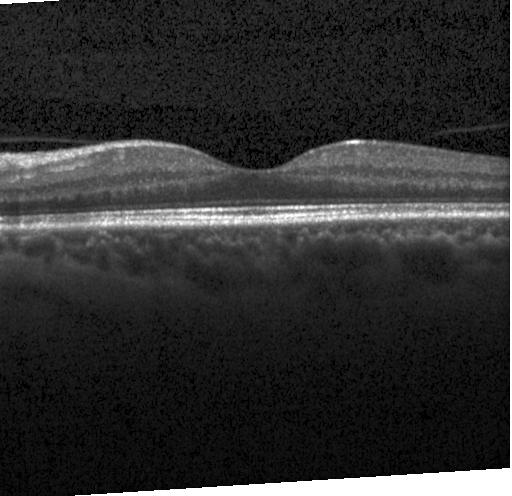

OCT B-scan showing no CNV, no DME, and no drusen.